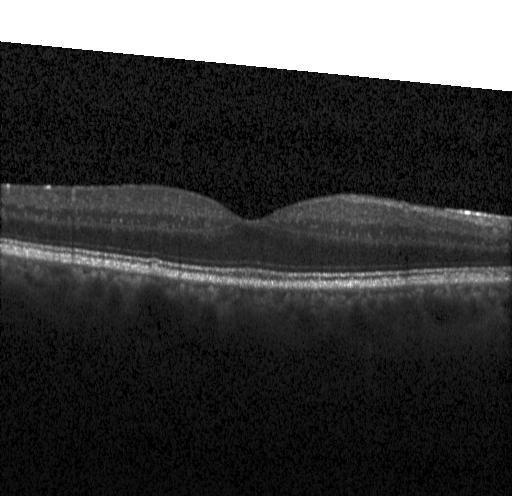
Neither CNV, DME, nor drusen.